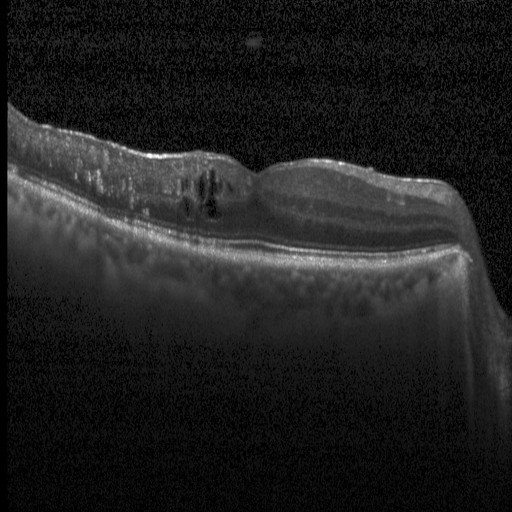

Retinal OCT cross-section. Heidelberg Spectralis. Diagnosis: diabetic macular edema.